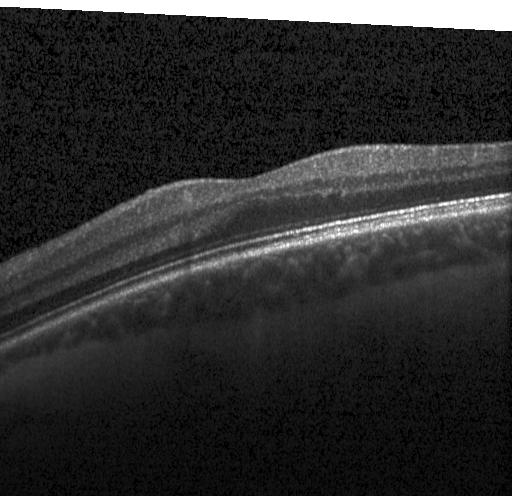

Spectral-domain OCT. OCT line scan. The scan shows no evidence of choroidal neovascularization, diabetic macular edema, or drusen.